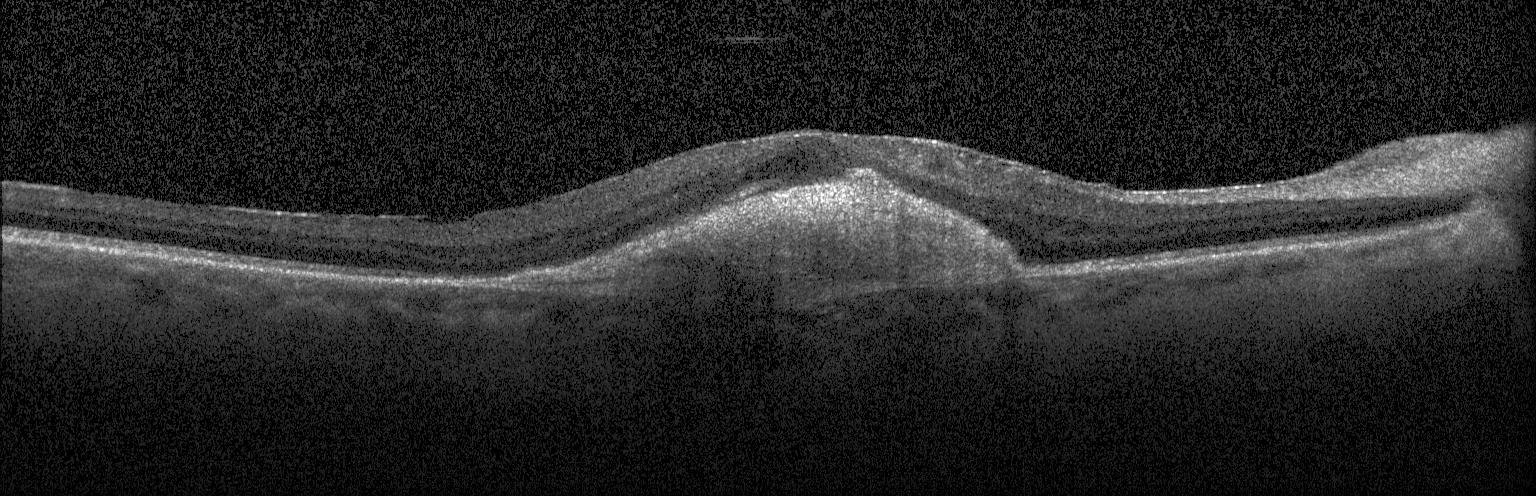
Acquired on a Heidelberg Spectralis; spectral-domain OCT; retinal OCT cross-section.
Diagnosis: a choroidal neovascular membrane.